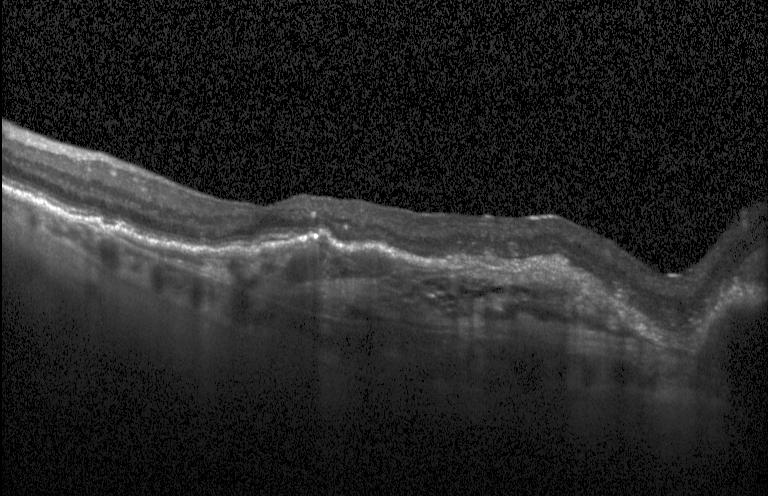 Spectral-domain OCT; Heidelberg Spectralis OCT system; retinal OCT cross-section.
Diagnosis: a choroidal neovascular membrane.